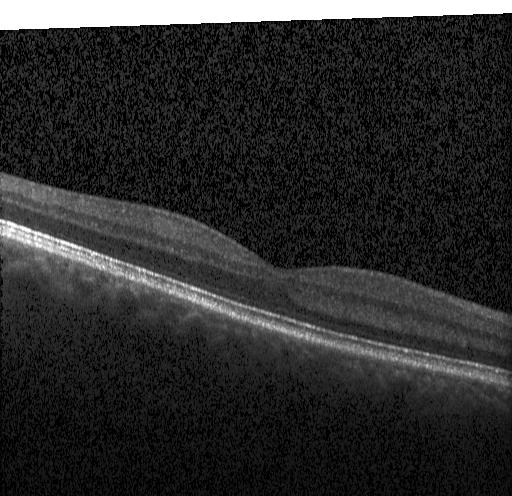 Impression: no CNV, DME, or drusen.